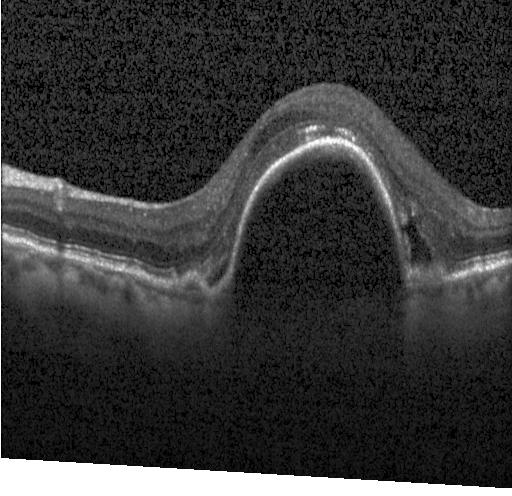
Finding: choroidal neovascularization (CNV).